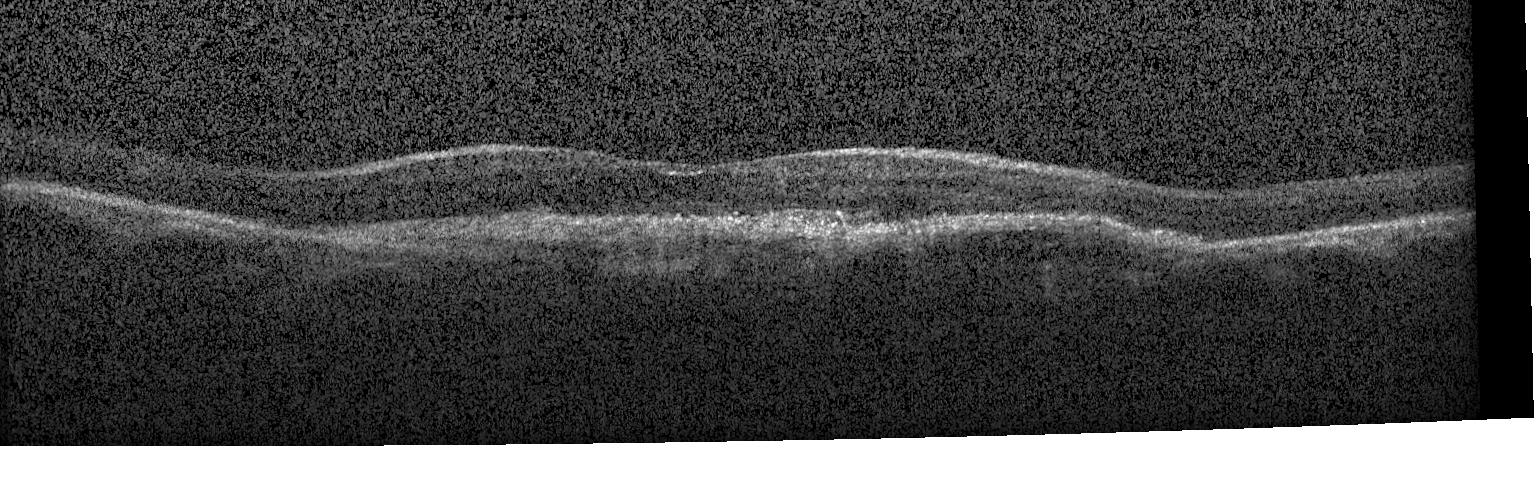 Centered on the fovea · retinal OCT B-scan · Heidelberg Spectralis OCT system — A choroidal neovascular membrane.